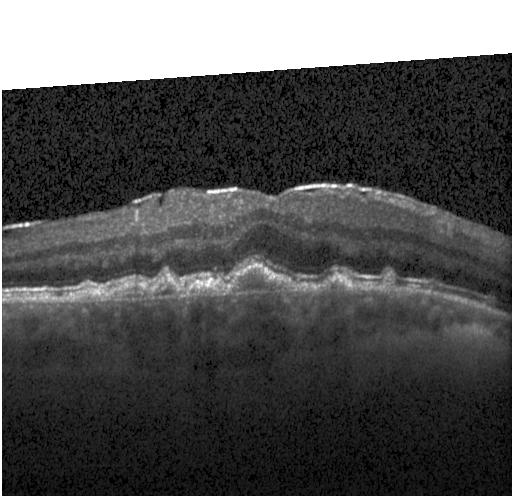
Optical coherence tomography B-scan. Assessment: a choroidal neovascular membrane.